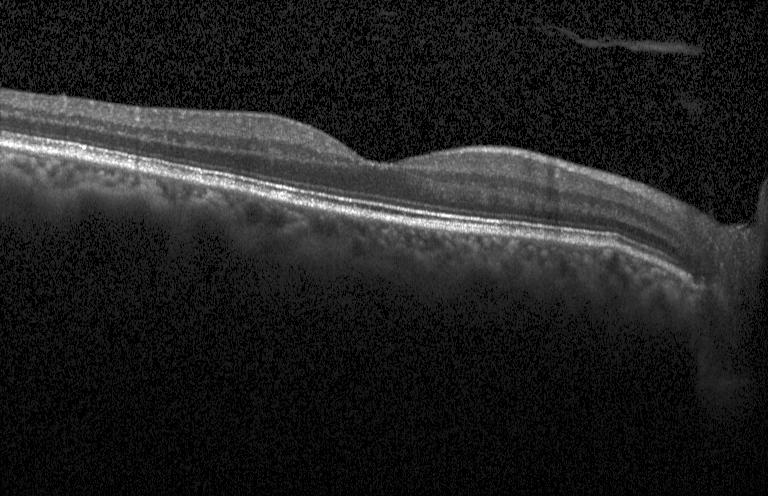 Optical coherence tomography scan. The scan shows no evidence of choroidal neovascularization, diabetic macular edema, or drusen.